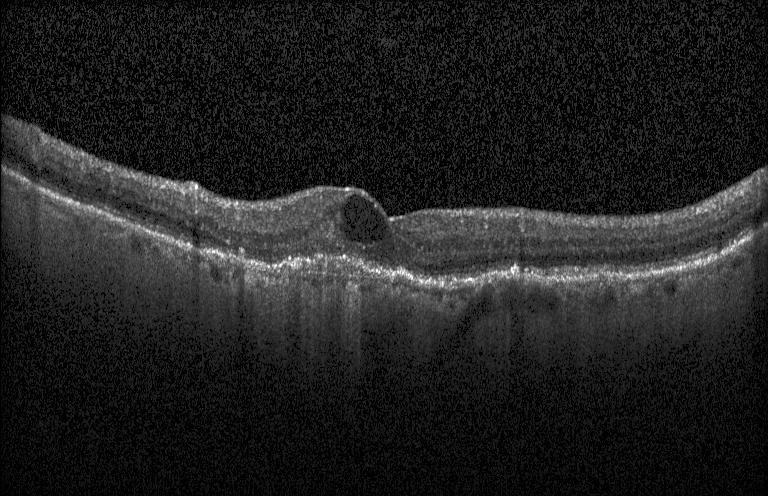 Heidelberg Spectralis. OCT line scan.
CNV.